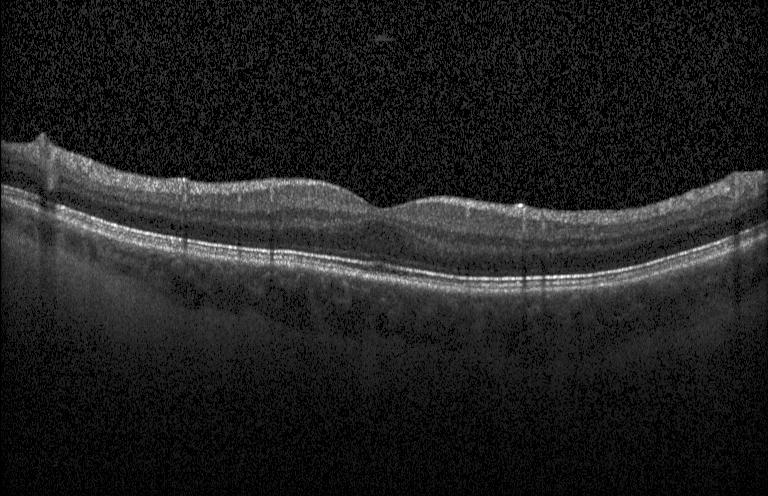 Optical coherence tomography B-scan; fovea-centered.
Diagnosis: no choroidal neovascularization, no diabetic macular edema, and no drusen.